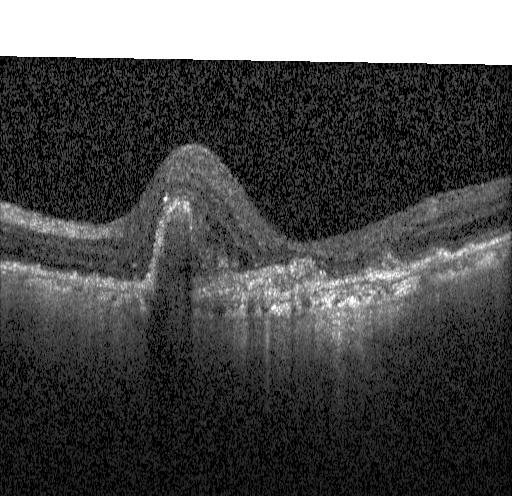 Macular OCT: a choroidal neovascular membrane.